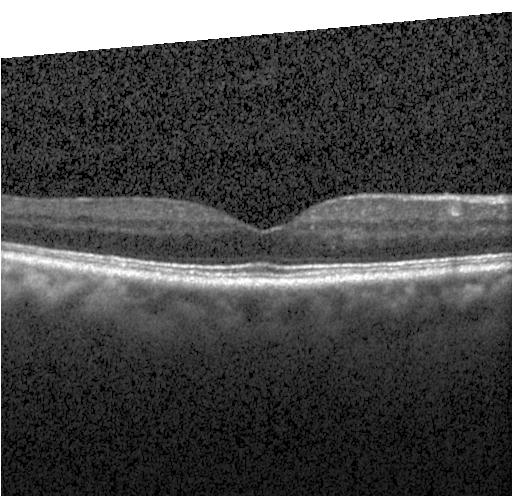
Retinal OCT B-scan
This B-scan demonstrates no choroidal neovascularization, diabetic macular edema, or drusen.